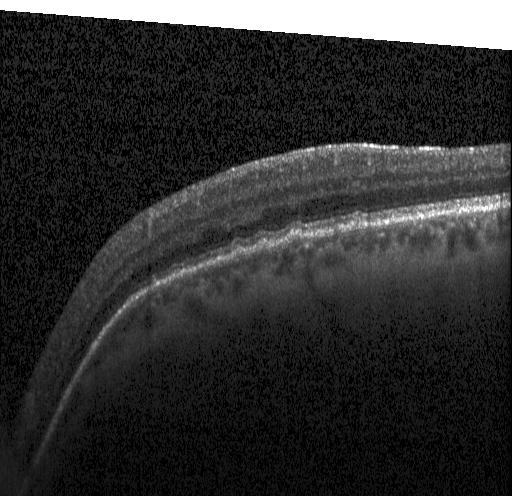

Macular OCT demonstrating sub-RPE drusenoid deposits.